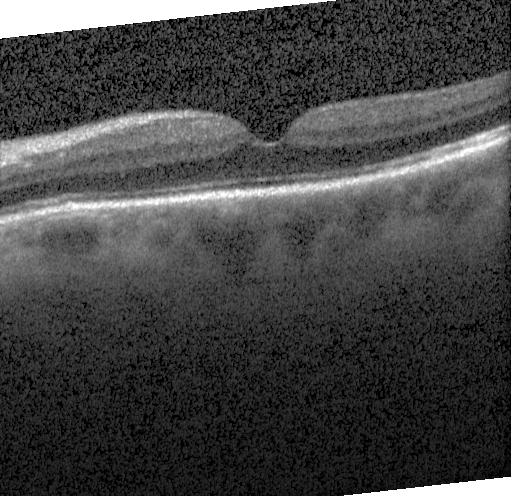 Instrument: Heidelberg Spectralis · retinal OCT cross-section
Diagnosis: neither CNV, DME, nor drusen.